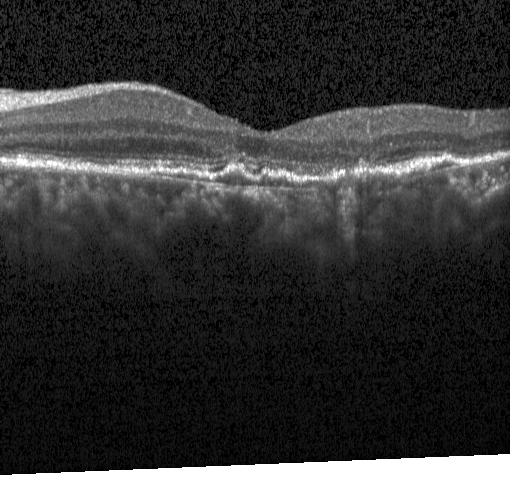

Impression: choroidal neovascularization (CNV).